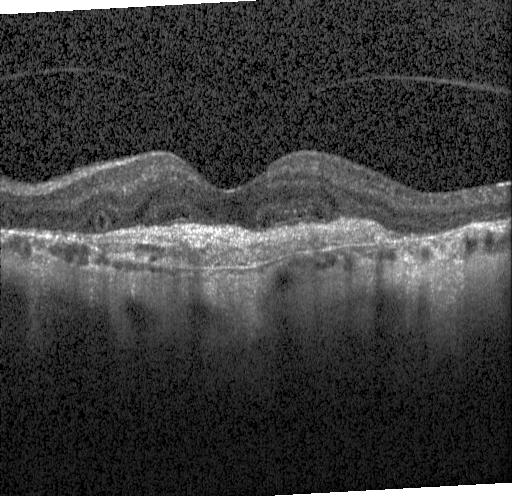 Optical coherence tomography B-scan
Dx: a choroidal neovascular membrane.